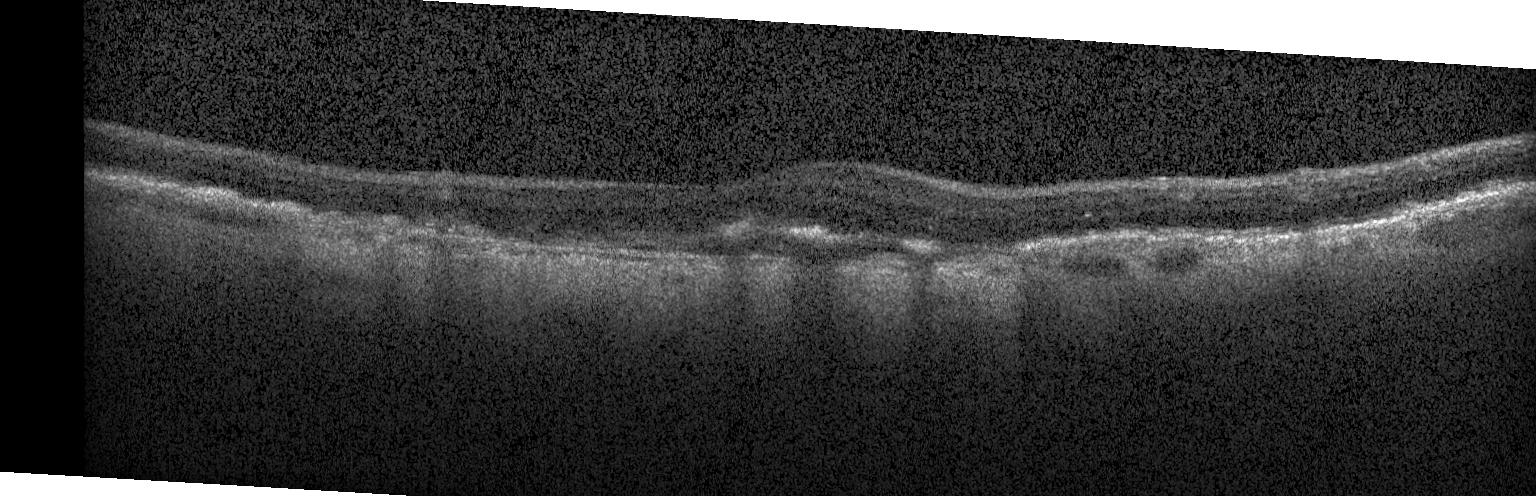

Retinal OCT B-scan, acquired on a Heidelberg Spectralis.
Impression: a choroidal neovascular membrane.